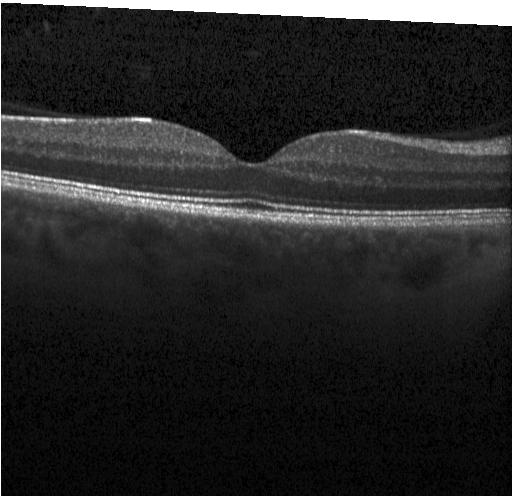
No choroidal neovascularization, no diabetic macular edema, and no drusen.